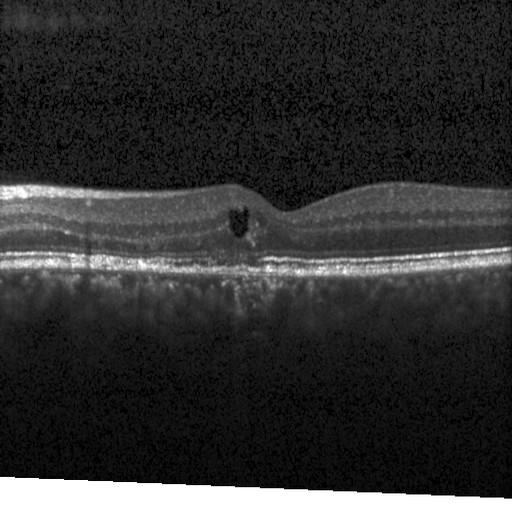 Retinal OCT B-scan, SD-OCT, instrument: Heidelberg Spectralis, centered on the fovea.
Finding: diabetic macular edema (DME).